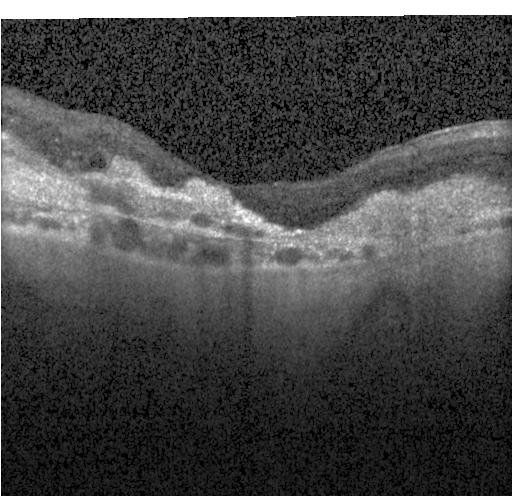
The scan shows choroidal neovascularization.